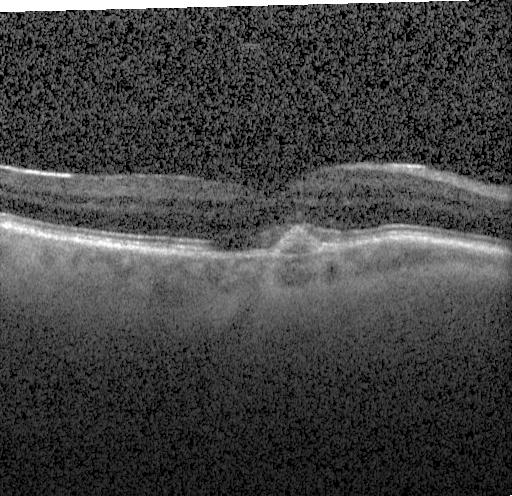
Finding: choroidal neovascularization.